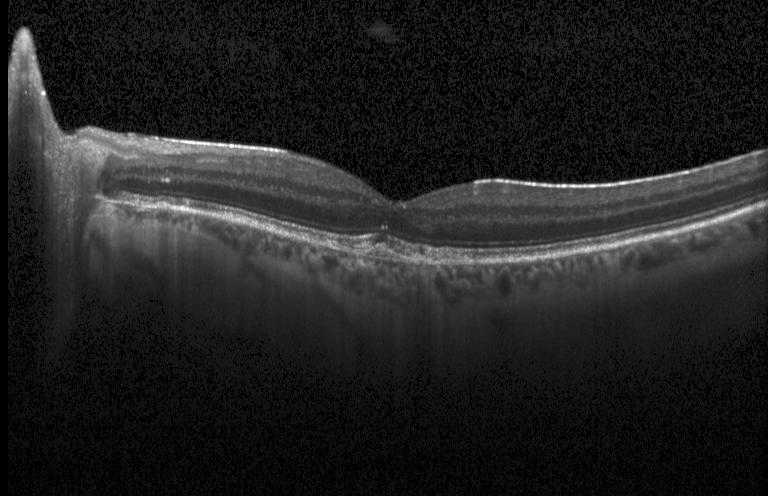

This B-scan demonstrates a choroidal neovascular membrane.